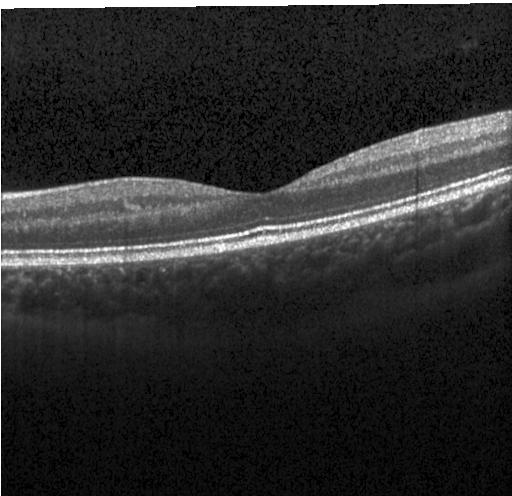 Instrument: Heidelberg Spectralis, retinal OCT B-scan — Finding: no evidence of choroidal neovascularization, diabetic macular edema, or drusen.